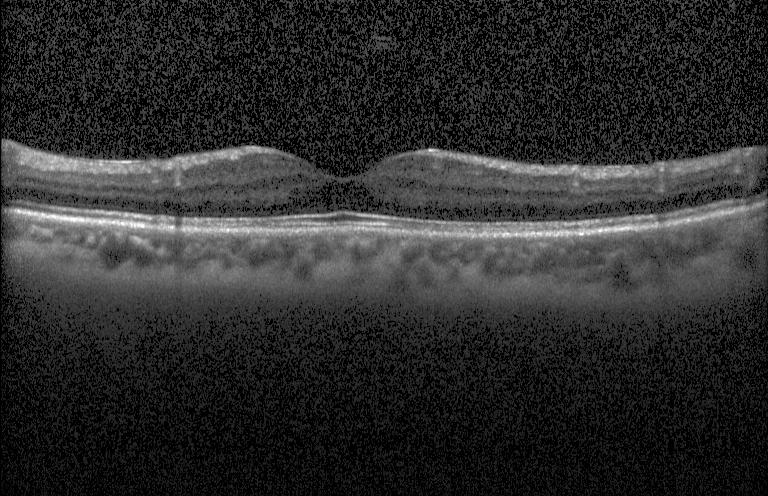 Retinal OCT cross-section. Through the macula. Spectral-domain OCT
OCT finding: no choroidal neovascularization, diabetic macular edema, or drusen.